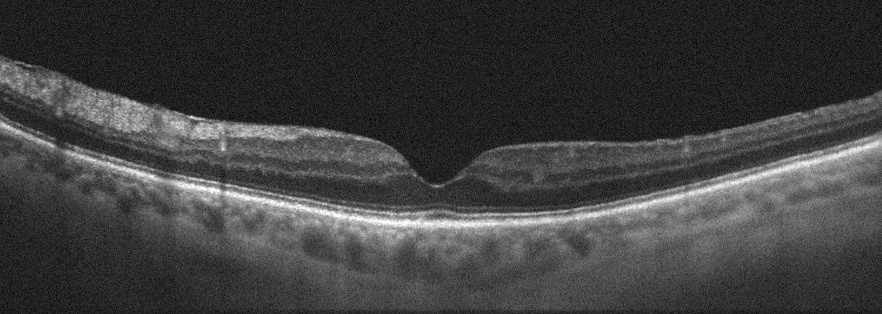
Through the macula · optical coherence tomography B-scan. Impression: retinal vein occlusion.